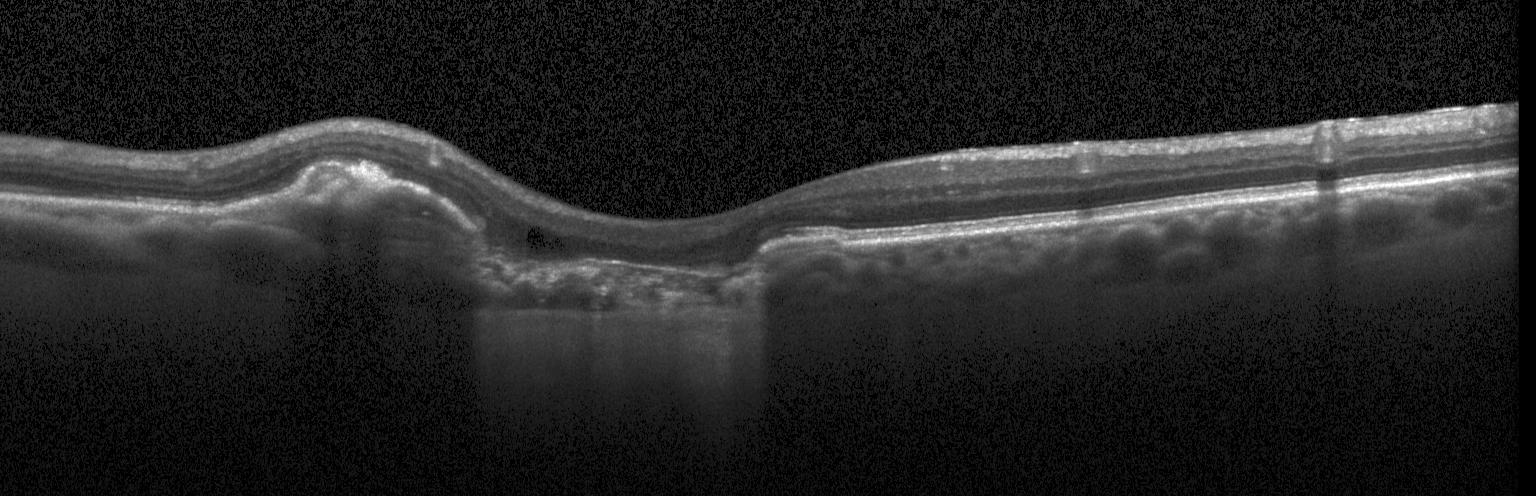

OCT line scan — Choroidal neovascularization.